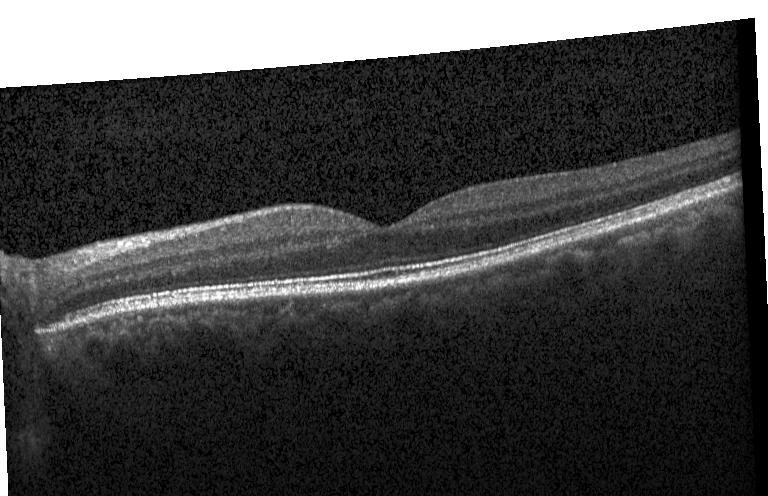

Retinal OCT cross-section, Heidelberg Spectralis. Impression: no choroidal neovascularization, diabetic macular edema, or drusen.